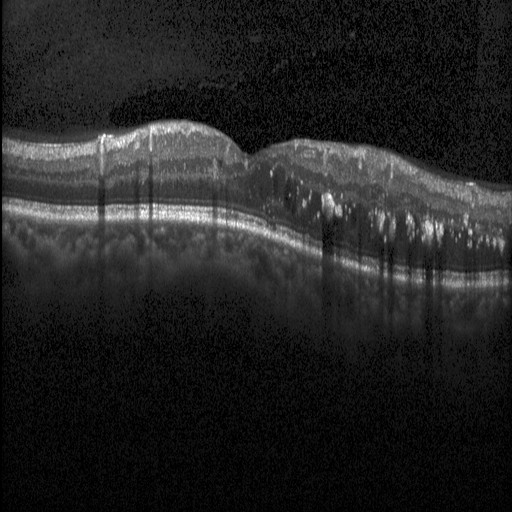

Through the macula. Retinal OCT B-scan. SD-OCT. Heidelberg Spectralis OCT system
Diagnosis: diabetic macular edema.